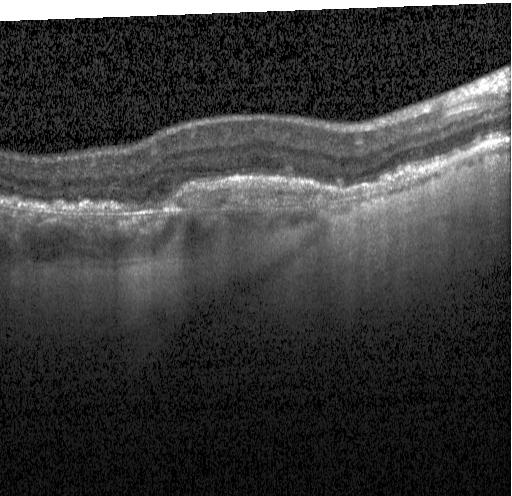

Impression: a choroidal neovascular membrane.